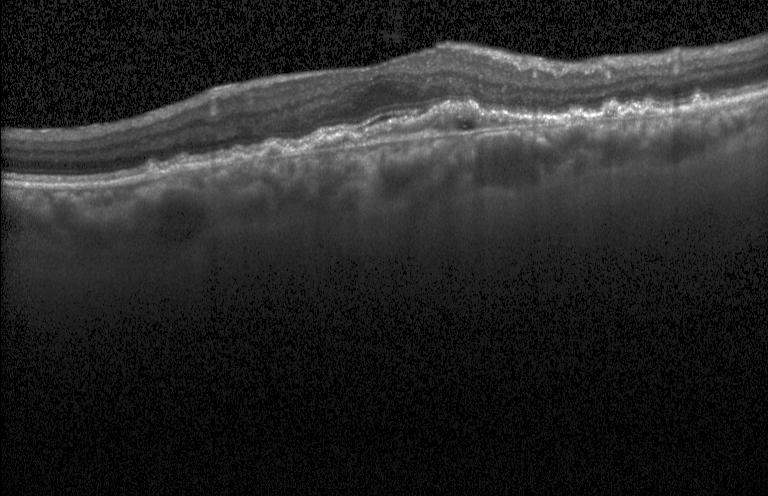 Macular scan. Optical coherence tomography scan. Dx: a choroidal neovascular membrane.